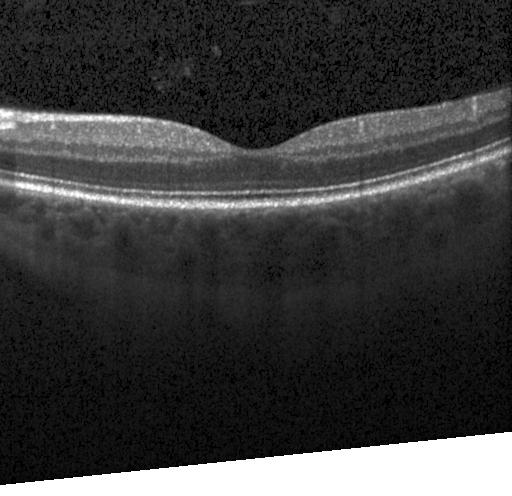

Retinal OCT cross-section
Assessment: no evidence of choroidal neovascularization, diabetic macular edema, or drusen.